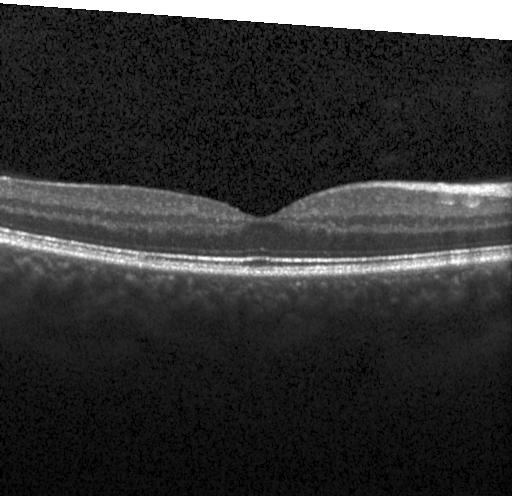

Optical coherence tomography scan
No evidence of CNV, DME, or drusen.